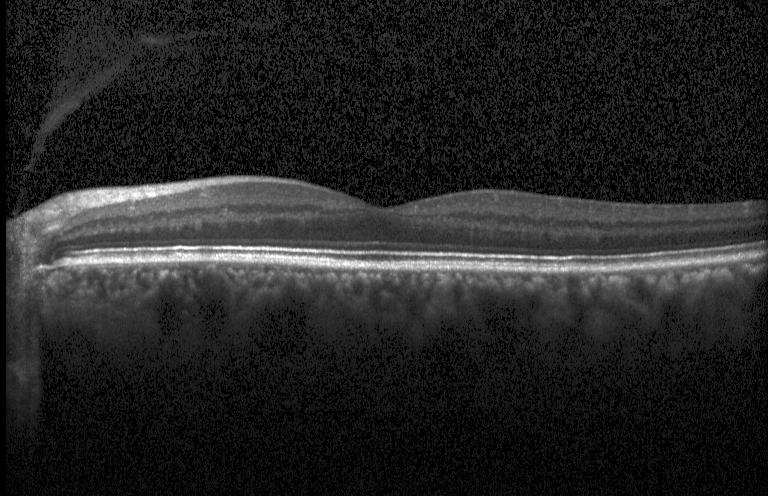 Spectral-domain OCT · instrument: Heidelberg Spectralis · retinal OCT B-scan · centered on the fovea
Impression: no evidence of choroidal neovascularization, diabetic macular edema, or drusen.